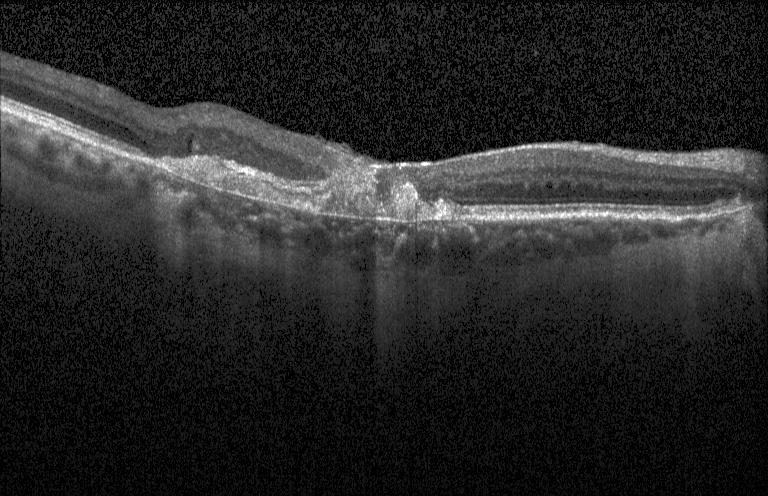
Diagnosis: a choroidal neovascular membrane.